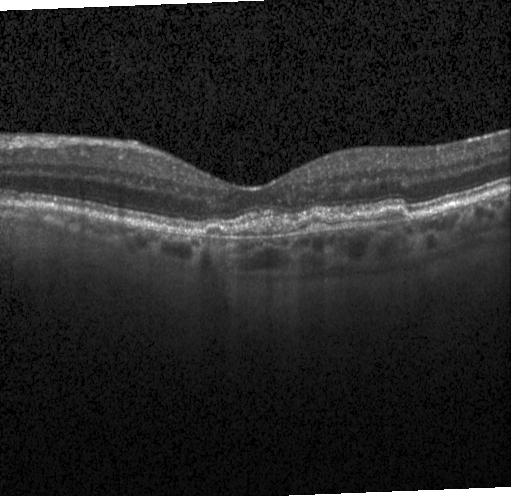

Macular OCT: choroidal neovascularization (CNV).